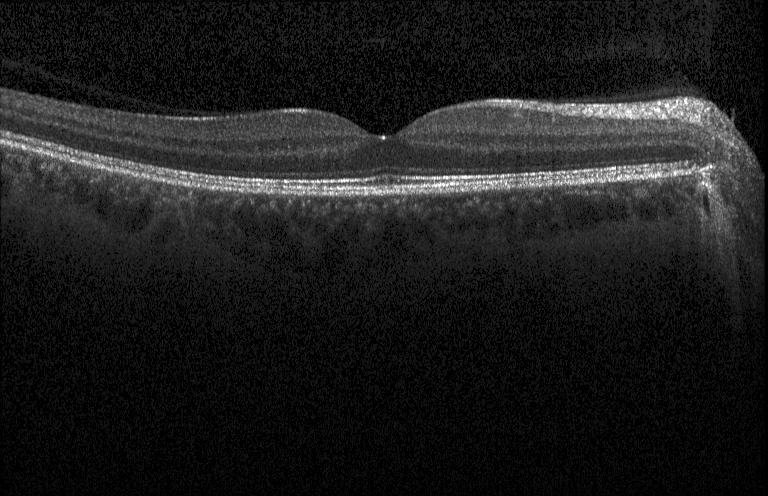 OCT B-scan, spectral-domain OCT, acquired on a Heidelberg Spectralis
Diagnosis: no choroidal neovascularization, no diabetic macular edema, and no drusen.